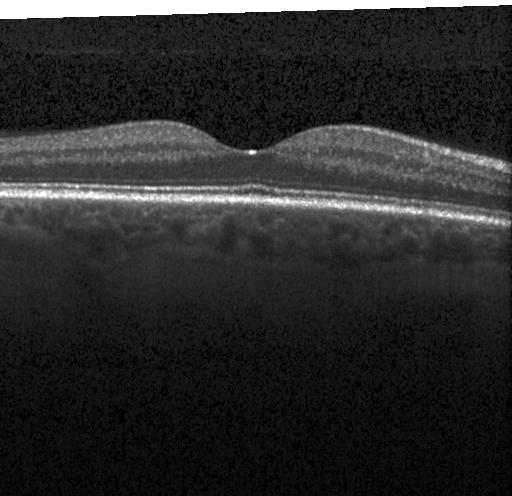

Horizontal scan through the fovea · retinal OCT B-scan · spectral-domain OCT · instrument: Heidelberg Spectralis — Diagnosis: no choroidal neovascularization, diabetic macular edema, or drusen.